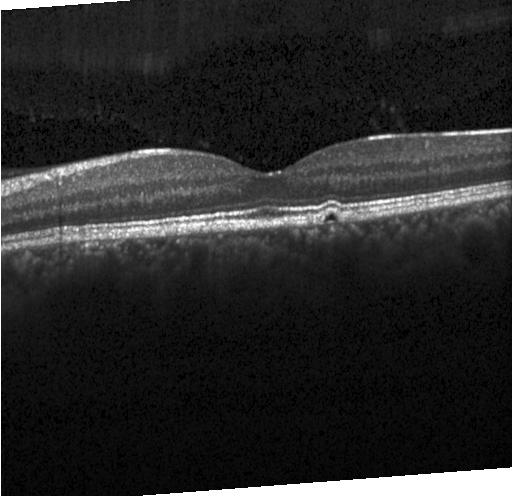

Horizontal scan through the fovea, OCT line scan
Dx: multiple drusen.